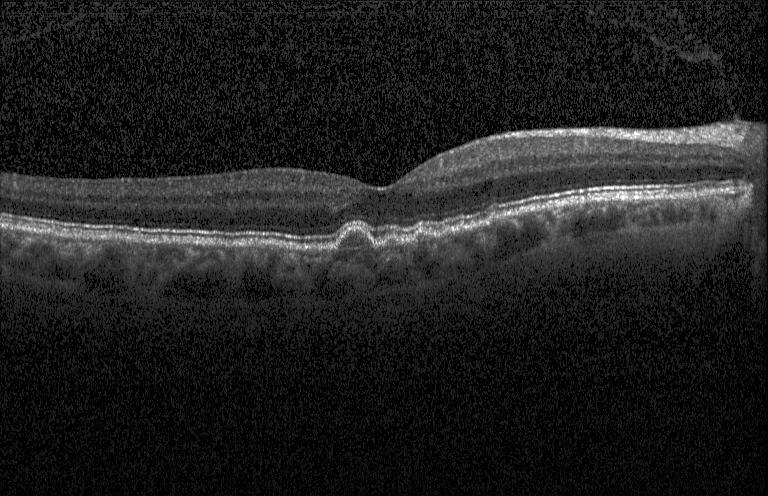

SD-OCT, OCT line scan. Impression: sub-RPE drusenoid deposits.